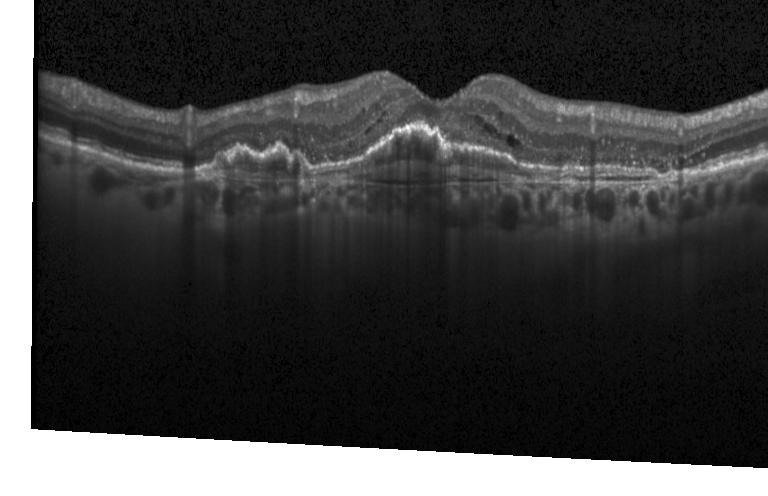 Retinal OCT B-scan · acquired on a Heidelberg Spectralis
The scan shows choroidal neovascularization (CNV).